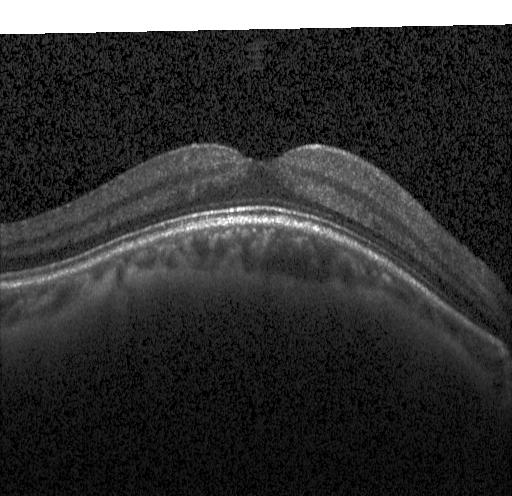
Spectral-domain OCT; fovea-centered; optical coherence tomography scan.
This B-scan demonstrates no choroidal neovascularization, diabetic macular edema, or drusen.